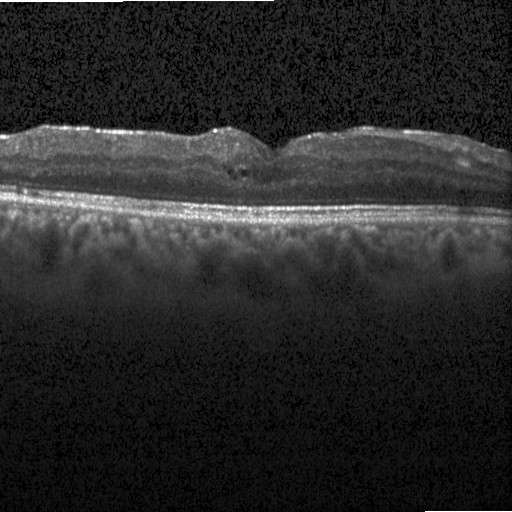

Macular OCT: diabetic macular edema.